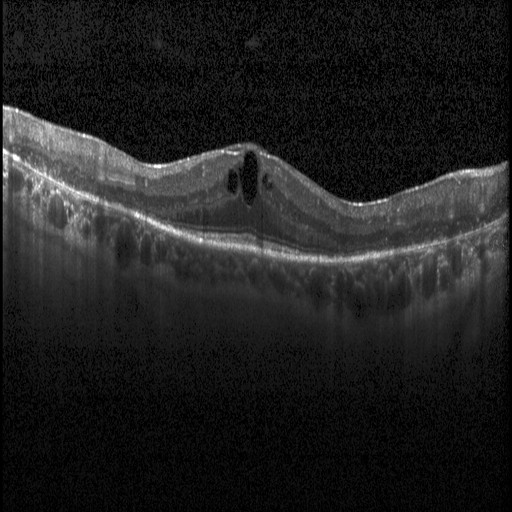
Impression: DME.